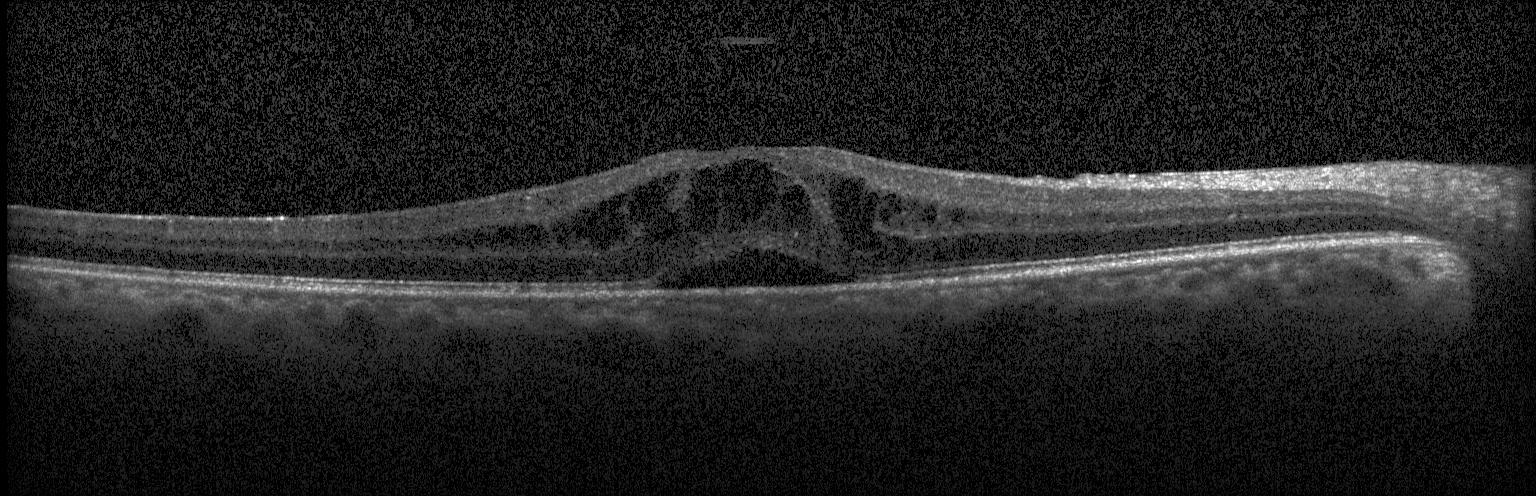 Spectral-domain OCT. Retinal OCT cross-section. Centered on the fovea. Instrument: Heidelberg Spectralis. OCT finding: diabetic macular edema (DME).